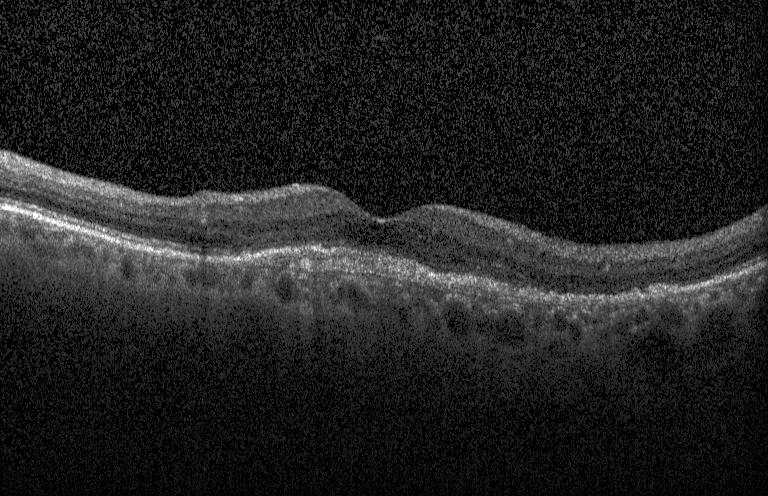

This B-scan demonstrates a choroidal neovascular membrane.